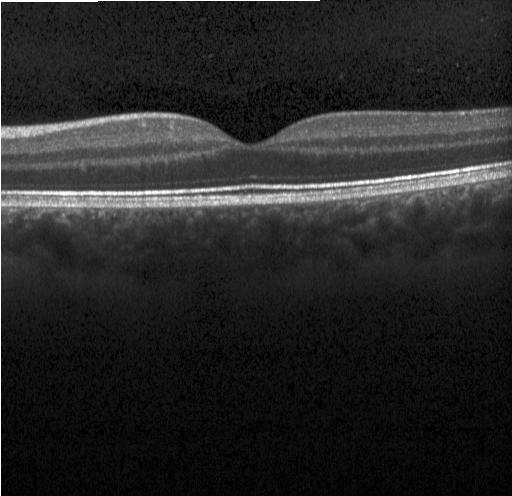
Through the macula, OCT B-scan, instrument: Heidelberg Spectralis. No choroidal neovascularization, diabetic macular edema, or drusen.